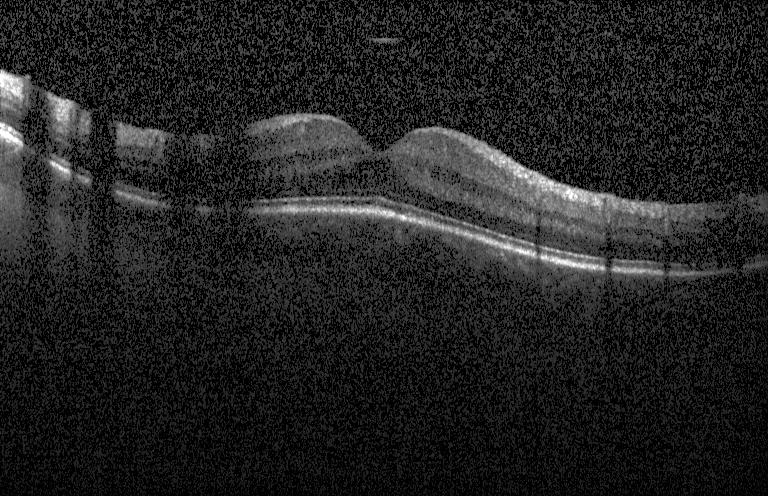
Optical coherence tomography B-scan · centered on the fovea — OCT finding: no evidence of choroidal neovascularization, diabetic macular edema, or drusen.